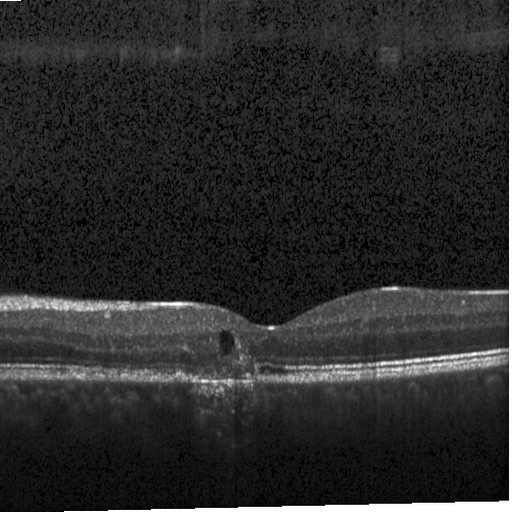

Optical coherence tomography B-scan. Horizontal scan through the fovea. Spectral-domain OCT
Macular OCT: diabetic macular edema.